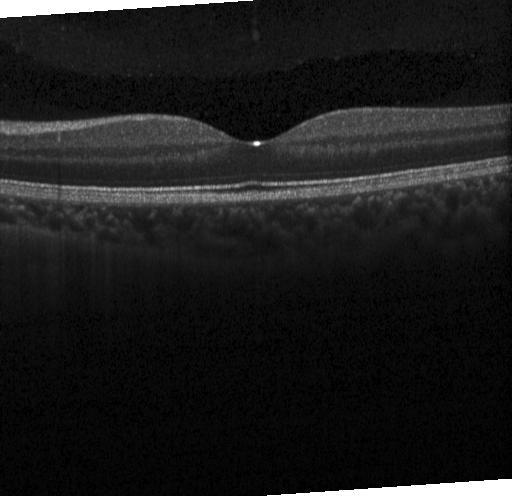 Impression: no choroidal neovascularization, no diabetic macular edema, and no drusen.